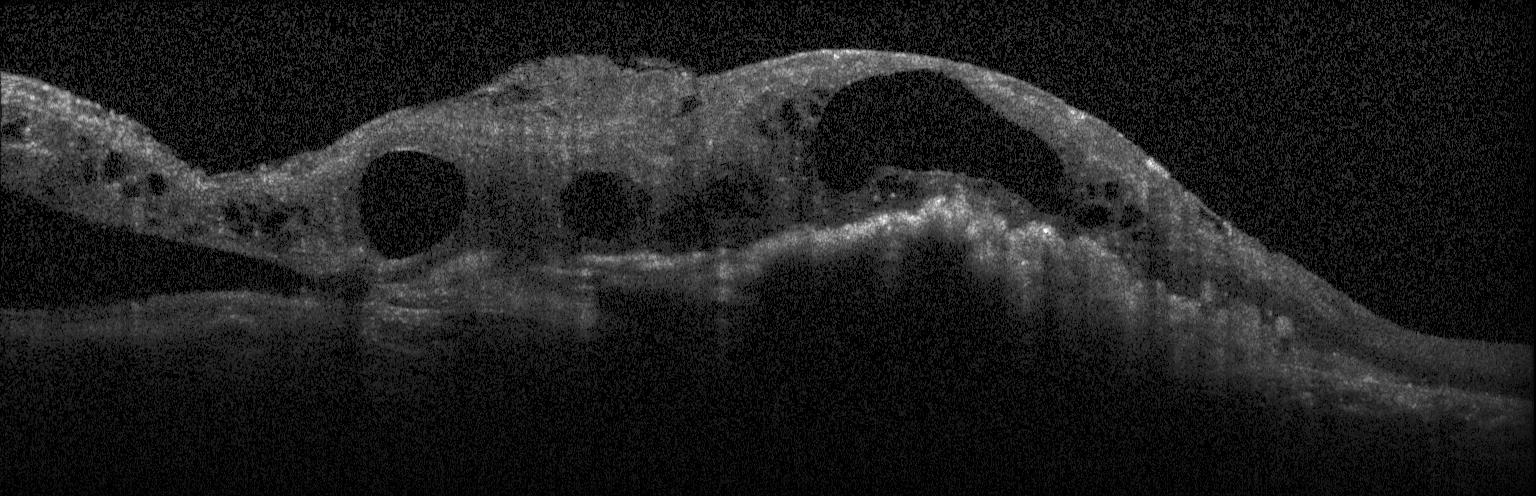 Impression: choroidal neovascularization (CNV).